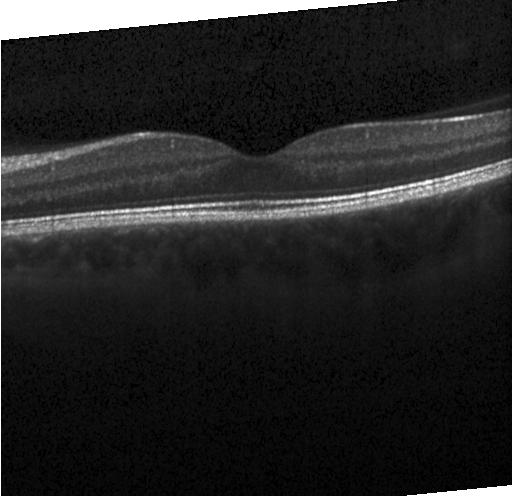

Centered on the fovea, SD-OCT, Heidelberg Spectralis, optical coherence tomography scan — Dx: no choroidal neovascularization, no diabetic macular edema, and no drusen.